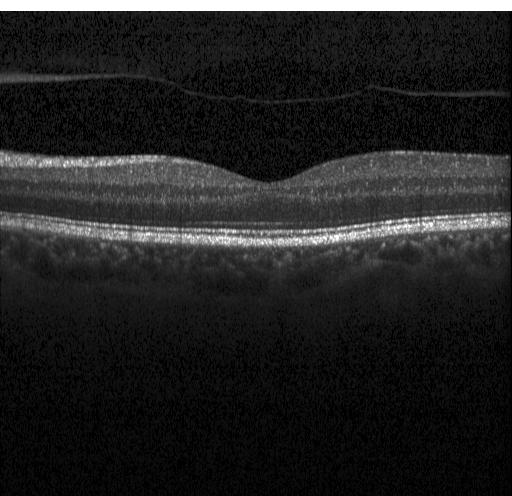
Diagnosis: no evidence of CNV, DME, or drusen.